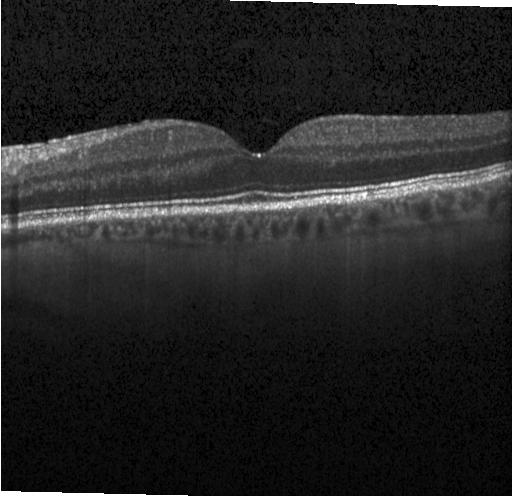
Finding: no choroidal neovascularization, diabetic macular edema, or drusen.